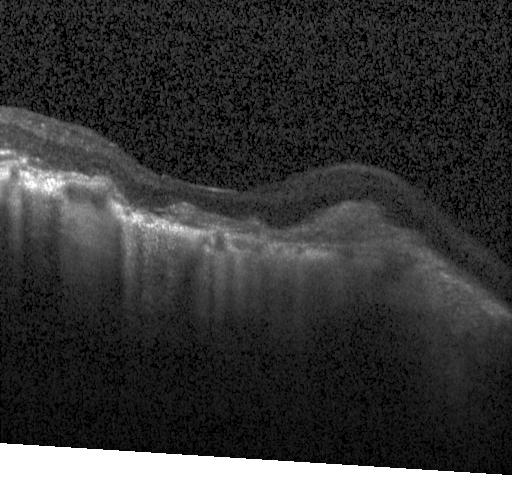 Retinal OCT cross-section showing choroidal neovascularization (CNV).